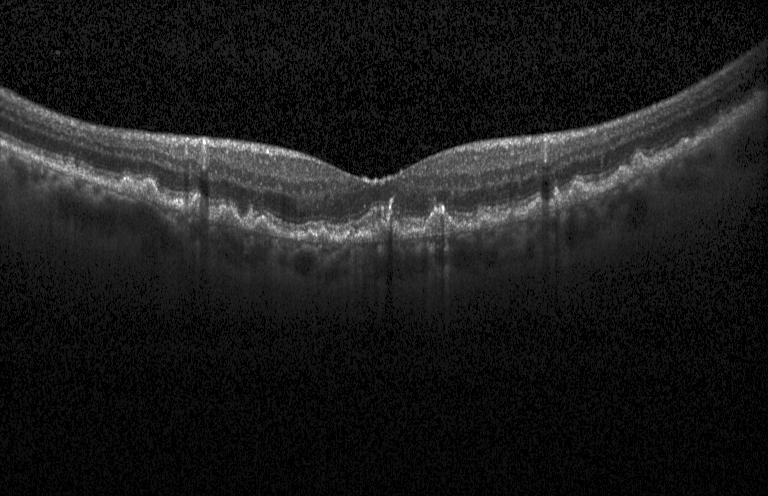
Heidelberg Spectralis OCT system, spectral-domain optical coherence tomography, through the macula, optical coherence tomography B-scan
Diagnosis: multiple drusen.